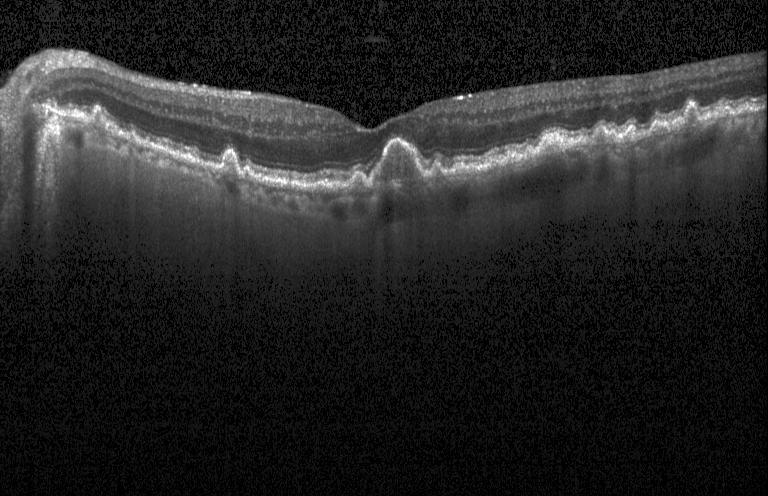 Diagnosis: sub-RPE drusenoid deposits.